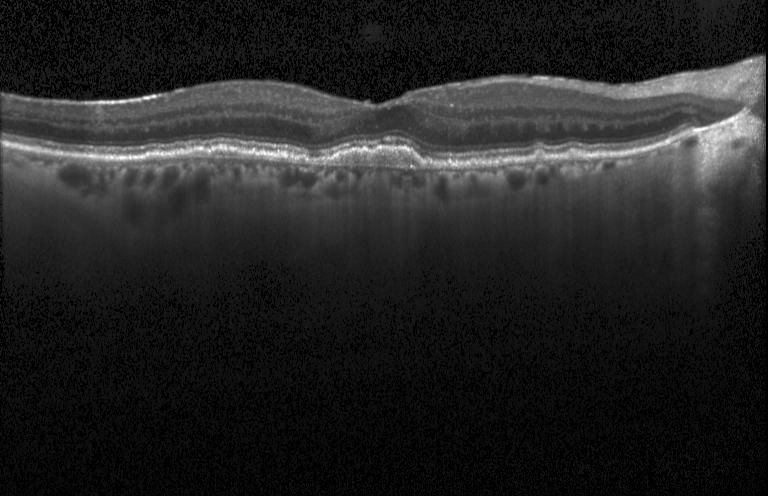

OCT line scan — Impression: a choroidal neovascular membrane.